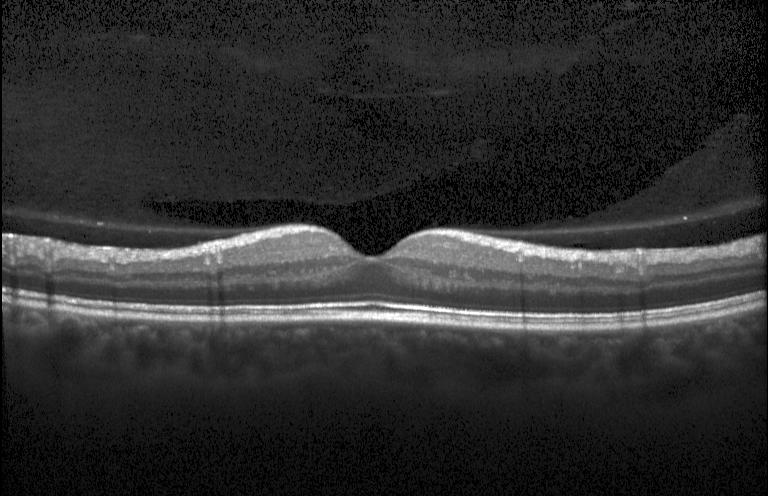

Retinal OCT B-scan.
Diagnosis: no evidence of CNV, DME, or drusen.